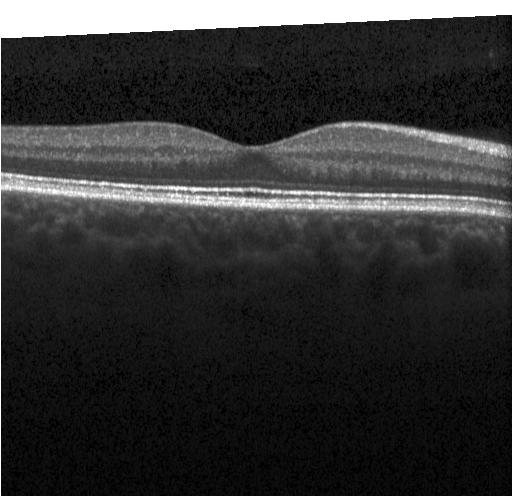 Spectral-domain optical coherence tomography; OCT B-scan; fovea-centered — Finding: no CNV, DME, or drusen.